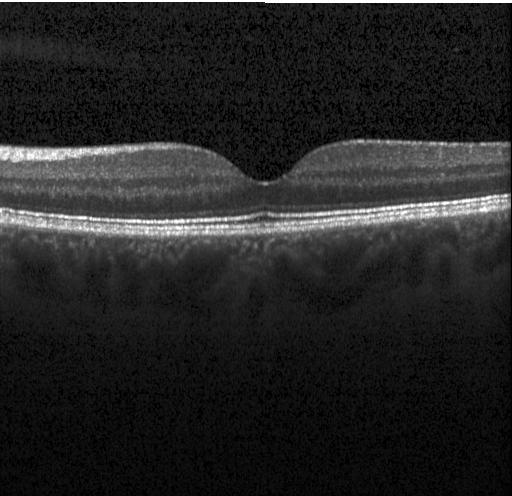

Retinal OCT cross-section, horizontal scan through the fovea, spectral-domain OCT. Impression: no evidence of CNV, DME, or drusen.